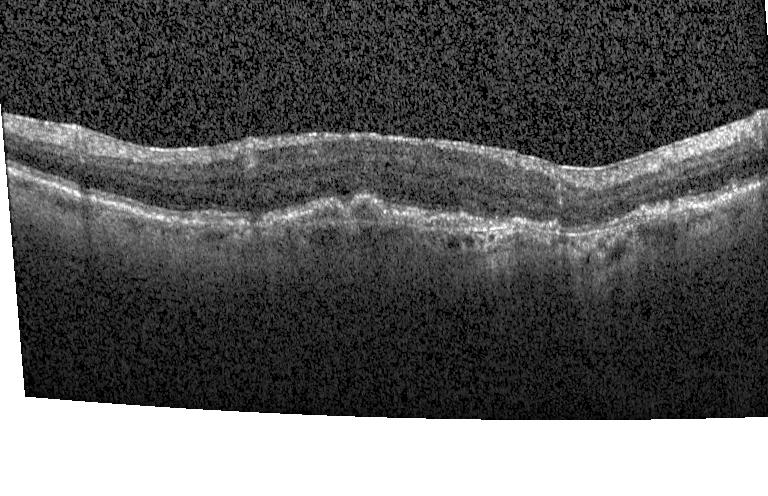
OCT scan showing a choroidal neovascular membrane.